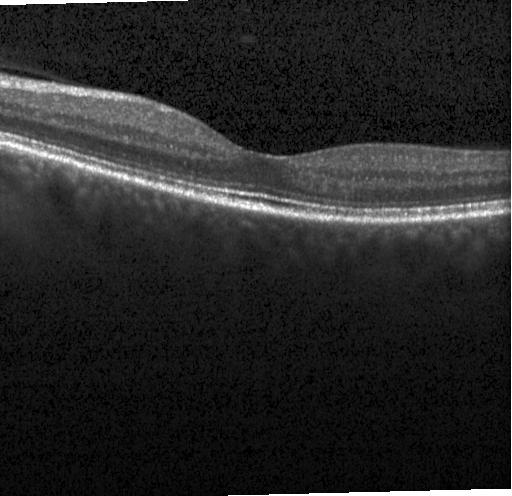
Retinal OCT B-scan, fovea-centered — Neither CNV, DME, nor drusen.